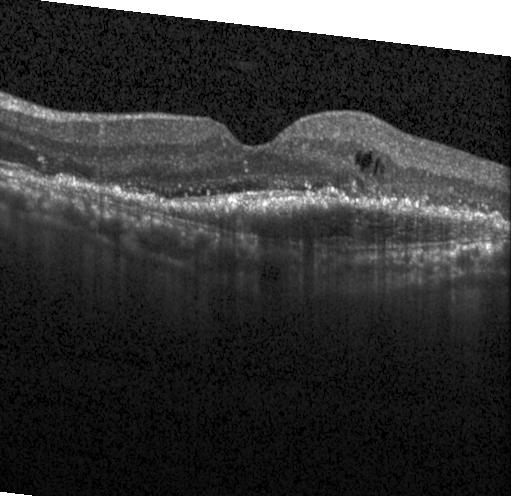
Through the macula; acquired on a Heidelberg Spectralis; OCT B-scan. Diagnosis: choroidal neovascularization.